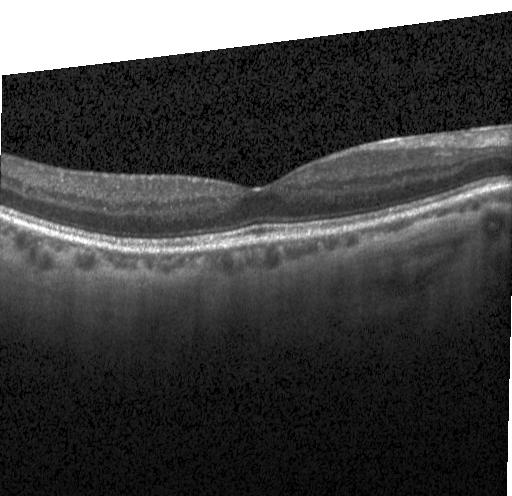
Impression: neither choroidal neovascularization, diabetic macular edema, nor drusen.